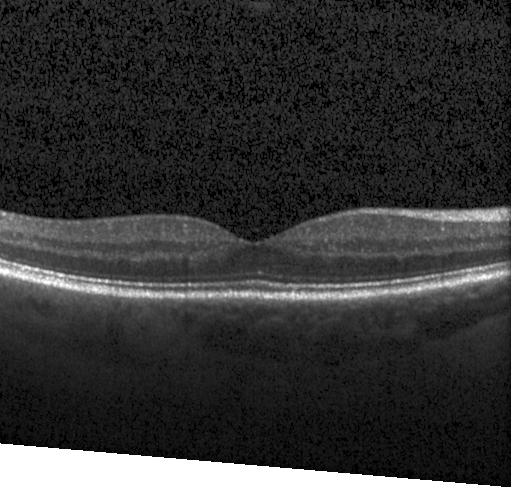
Macular OCT demonstrating no evidence of choroidal neovascularization, diabetic macular edema, or drusen.